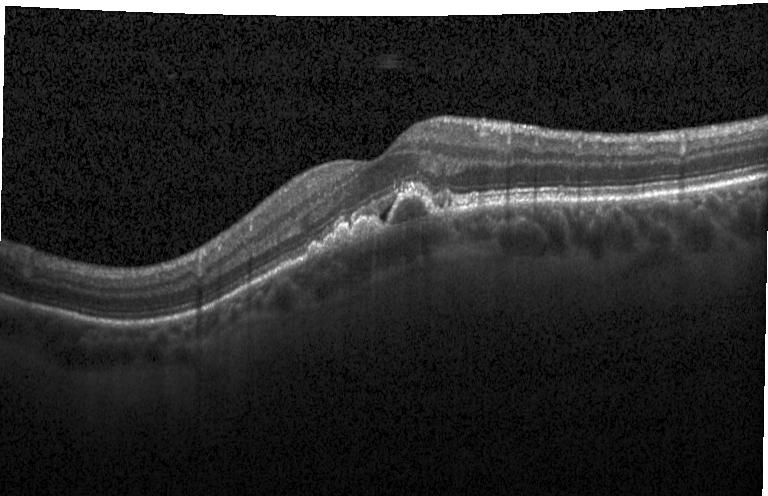
Spectral-domain OCT · optical coherence tomography scan. Impression: a choroidal neovascular membrane.